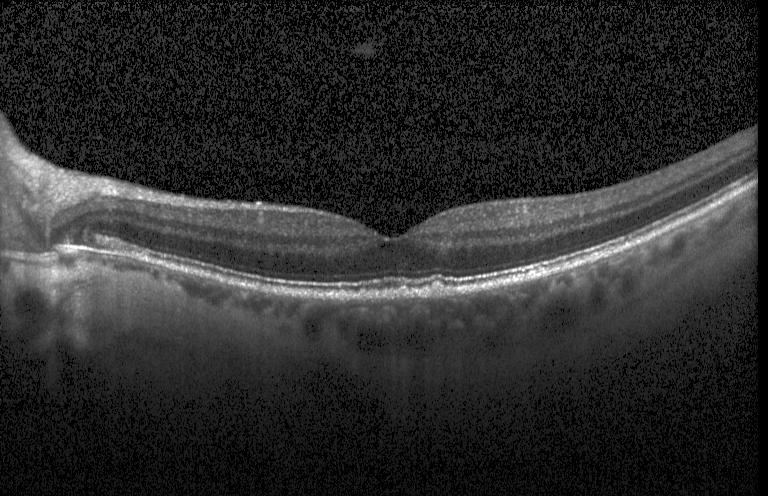

Heidelberg Spectralis OCT system, OCT B-scan, SD-OCT.
This B-scan demonstrates drusen.